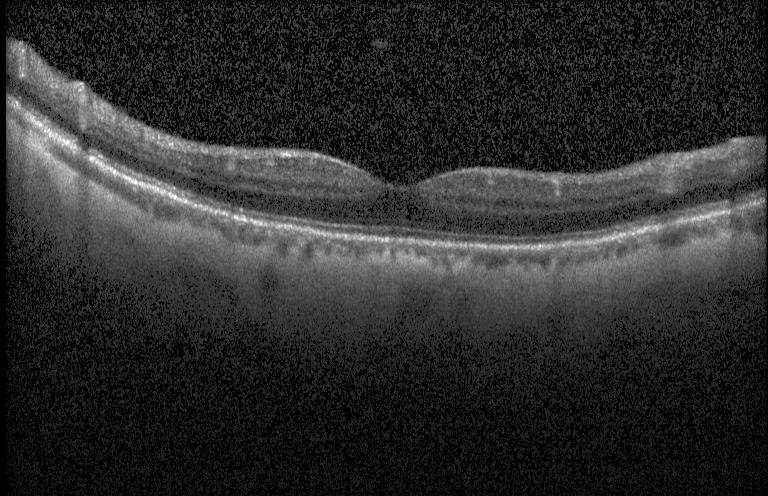 Instrument: Heidelberg Spectralis; retinal OCT cross-section; spectral-domain optical coherence tomography; centered on the fovea
This B-scan demonstrates no choroidal neovascularization, diabetic macular edema, or drusen.